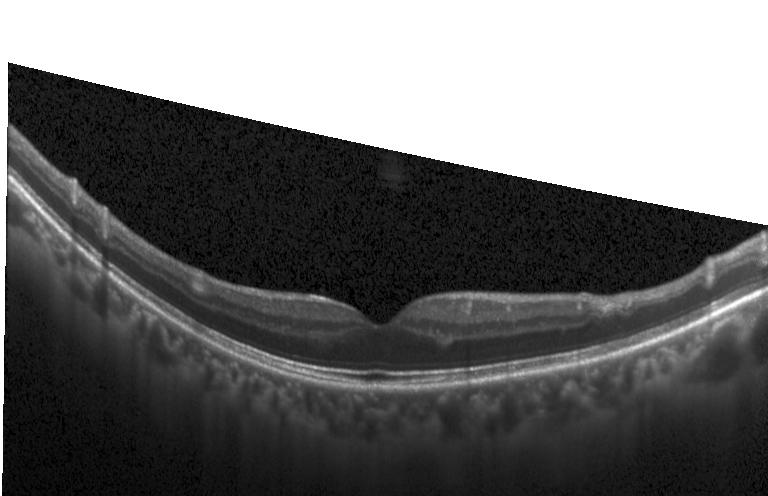

Impression: neither choroidal neovascularization, diabetic macular edema, nor drusen.